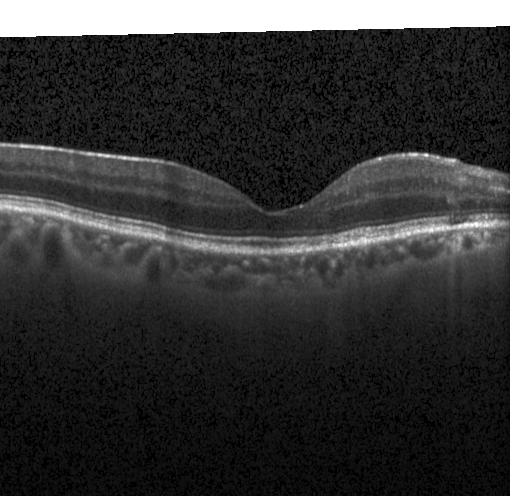

The scan shows no evidence of choroidal neovascularization, diabetic macular edema, or drusen.